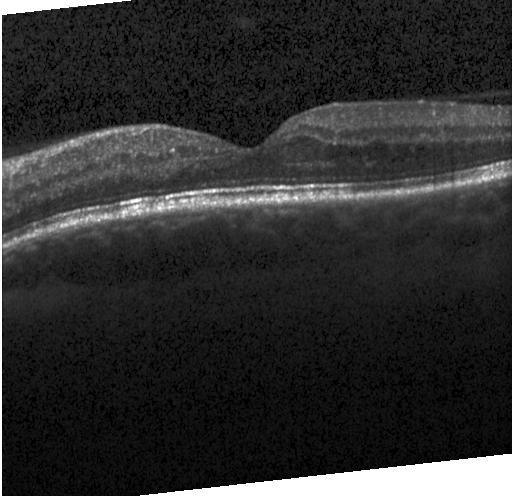
Heidelberg Spectralis; optical coherence tomography scan; spectral-domain OCT — Macular OCT: DME.